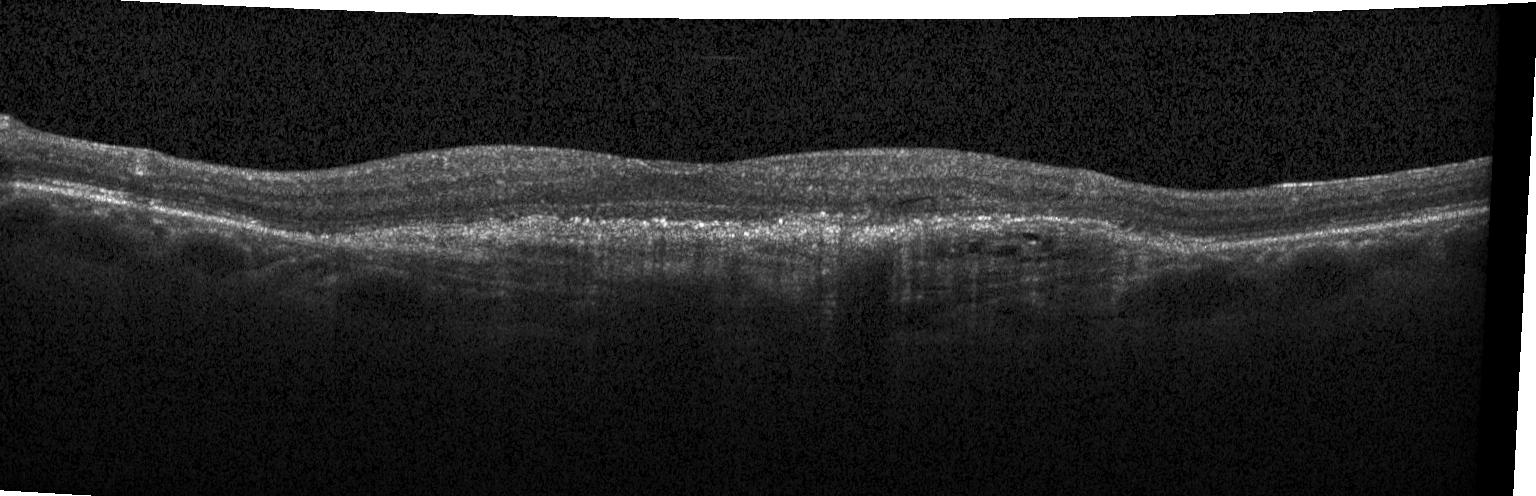
Macular scan. Acquired on a Heidelberg Spectralis. Optical coherence tomography B-scan. Spectral-domain optical coherence tomography.
Finding: choroidal neovascularization.